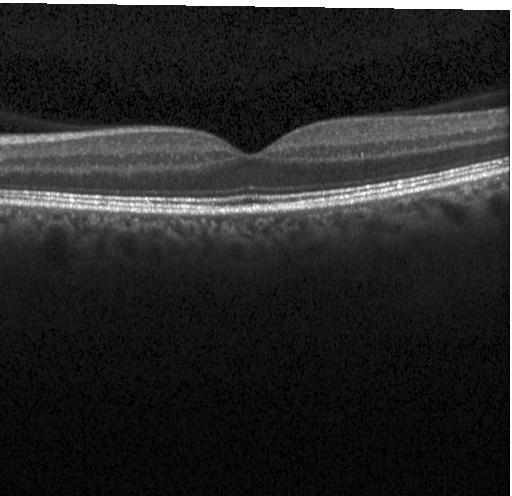
Instrument: Heidelberg Spectralis · optical coherence tomography B-scan · spectral-domain optical coherence tomography.
Assessment: neither choroidal neovascularization, diabetic macular edema, nor drusen.